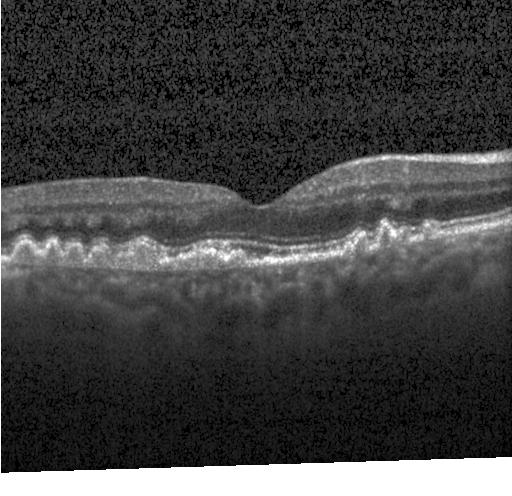 Dx: sub-RPE drusenoid deposits.